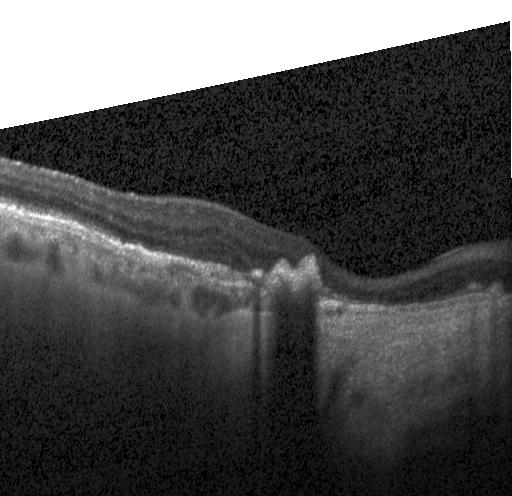 Instrument: Heidelberg Spectralis; OCT B-scan. This B-scan demonstrates a choroidal neovascular membrane.